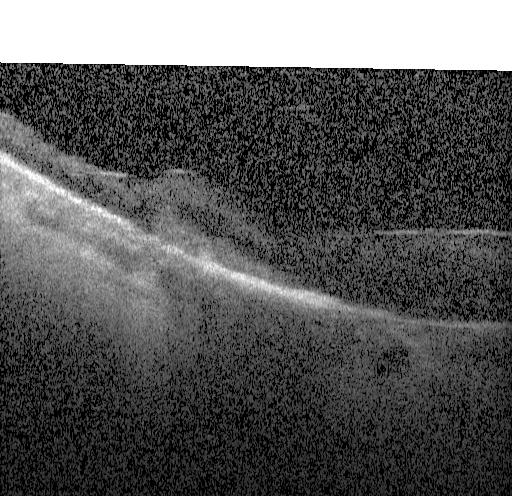

Retinal OCT cross-section; spectral-domain OCT; fovea-centered
Finding: a choroidal neovascular membrane.